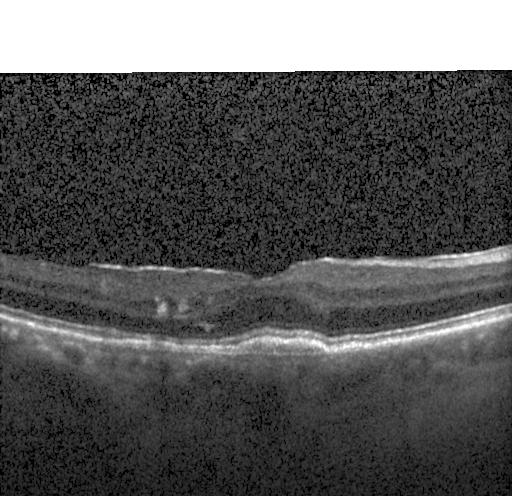 Dx: choroidal neovascularization (CNV).